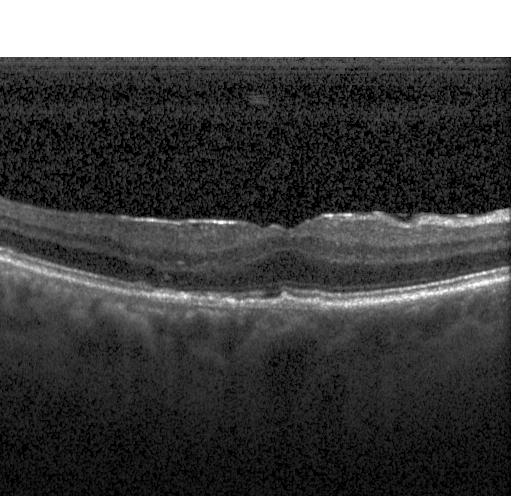
OCT B-scan
This B-scan demonstrates choroidal neovascularization.